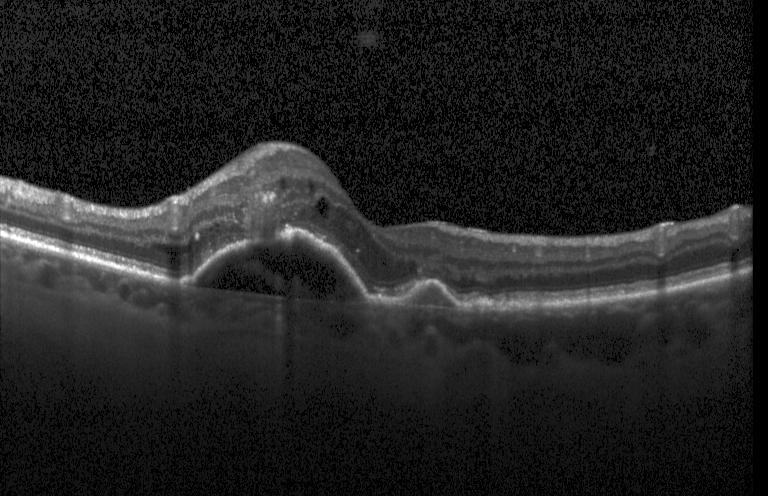
Heidelberg Spectralis; macular scan; spectral-domain optical coherence tomography; OCT B-scan
Finding: a choroidal neovascular membrane.